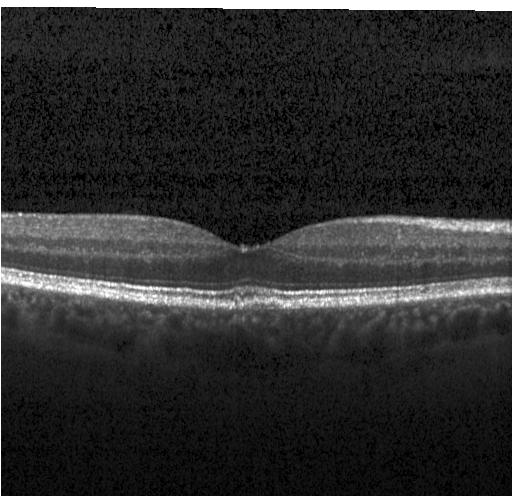

Macular OCT demonstrating drusen.